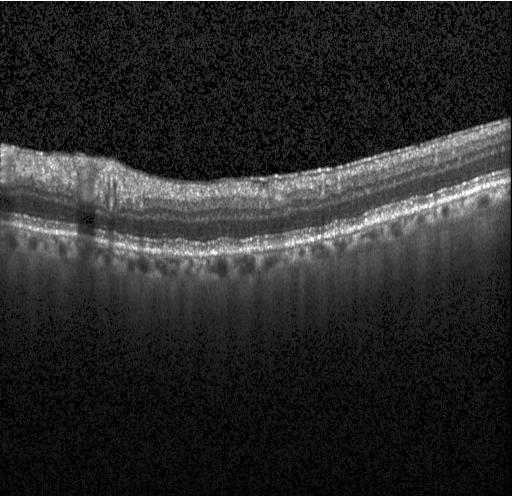 Retinal OCT cross-section.
Impression: sub-RPE drusenoid deposits.